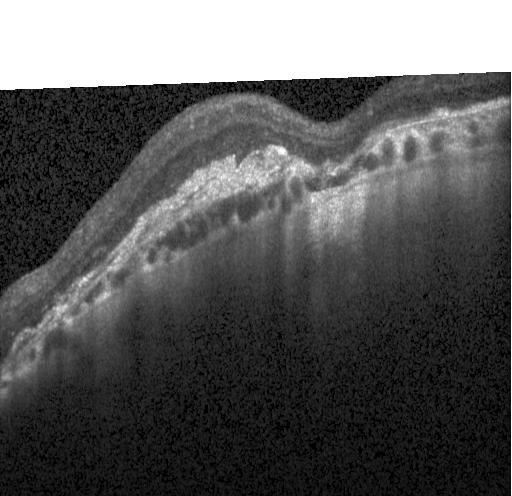 Optical coherence tomography B-scan.
The scan shows a choroidal neovascular membrane.